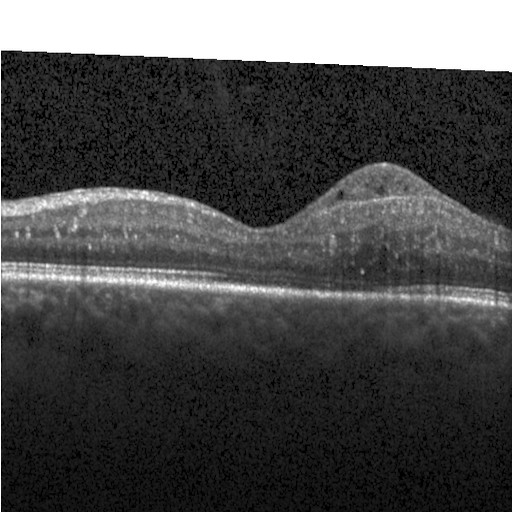
OCT finding: diabetic macular edema (DME).